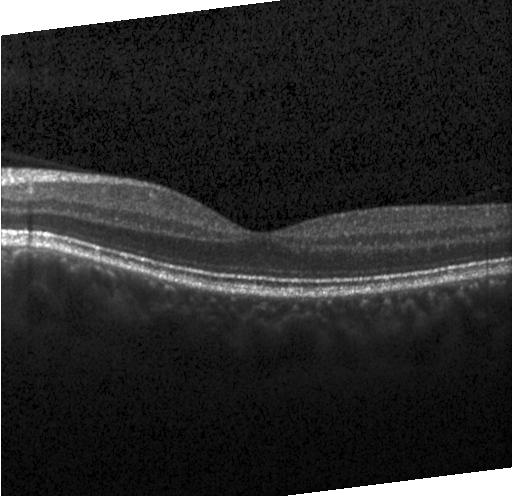 Macular OCT: no choroidal neovascularization, diabetic macular edema, or drusen.